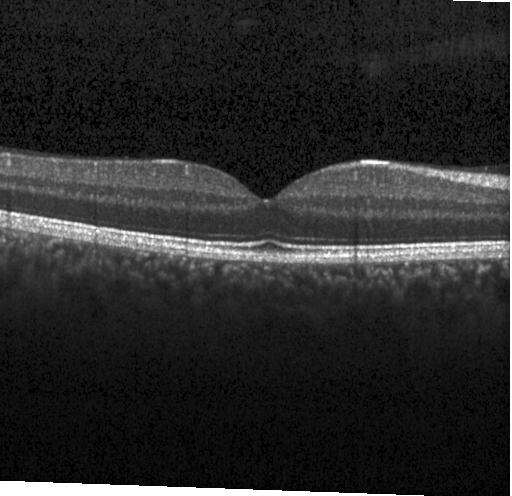
Spectral-domain OCT B-scan: no choroidal neovascularization, no diabetic macular edema, and no drusen.